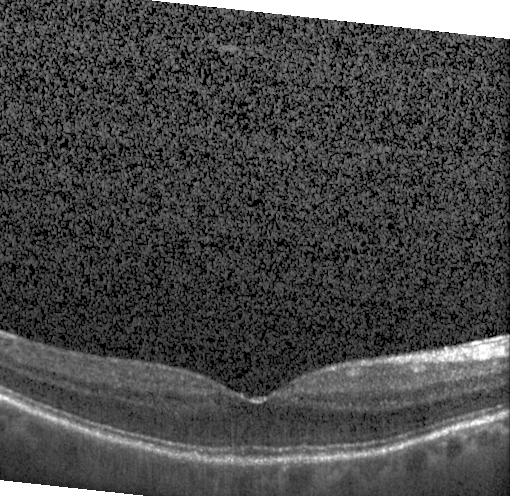

Neither choroidal neovascularization, diabetic macular edema, nor drusen.